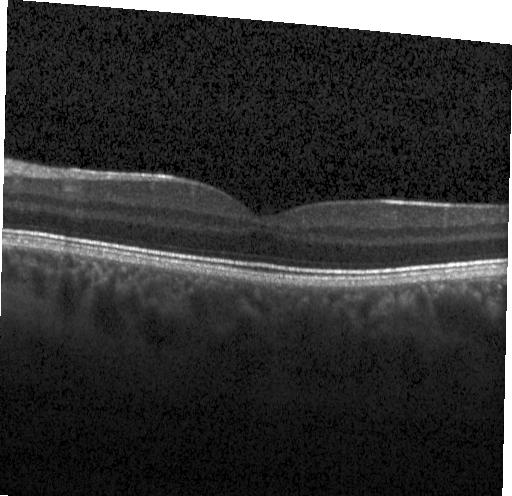
Assessment: no evidence of CNV, DME, or drusen.